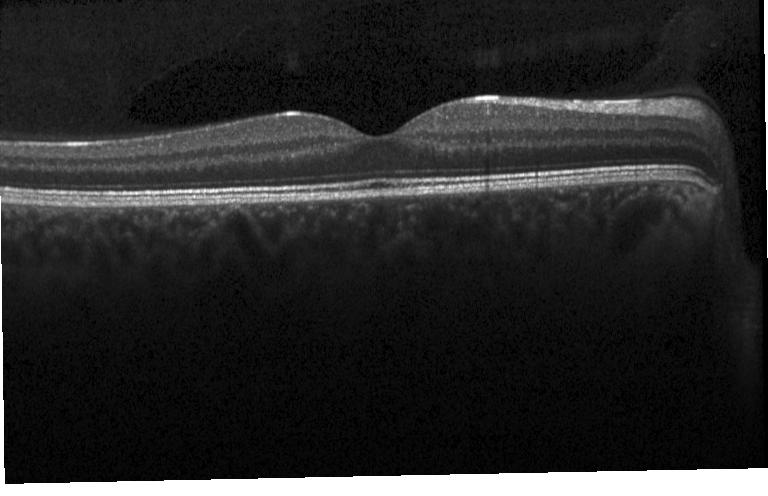 Impression: no choroidal neovascularization, diabetic macular edema, or drusen.